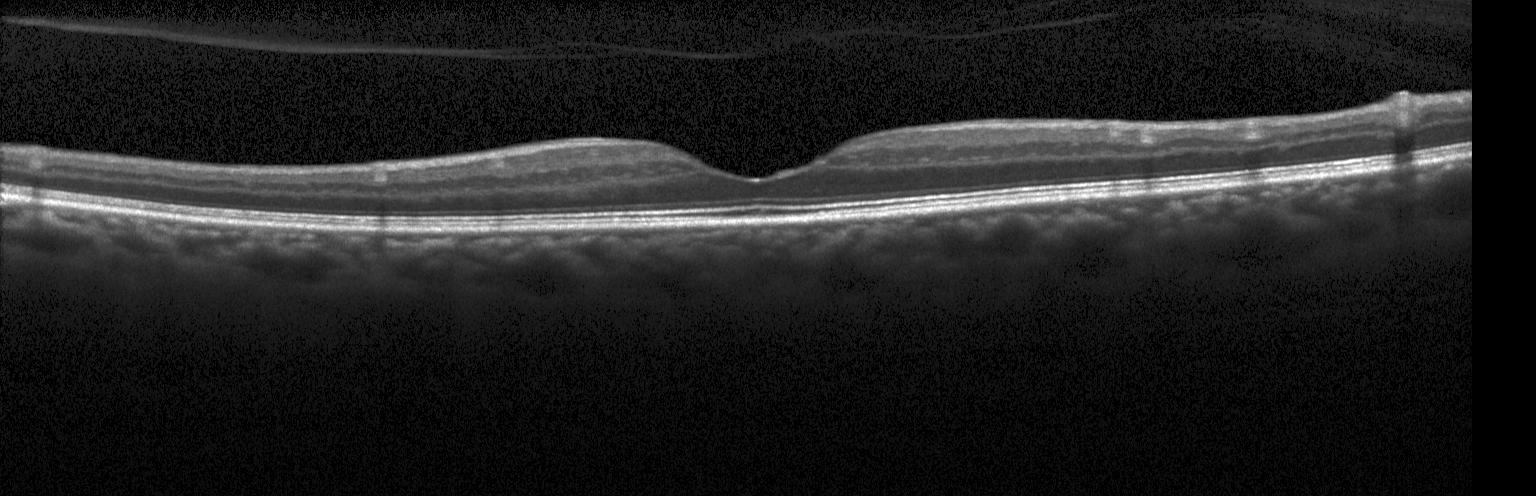 Spectral-domain OCT B-scan: neither CNV, DME, nor drusen.